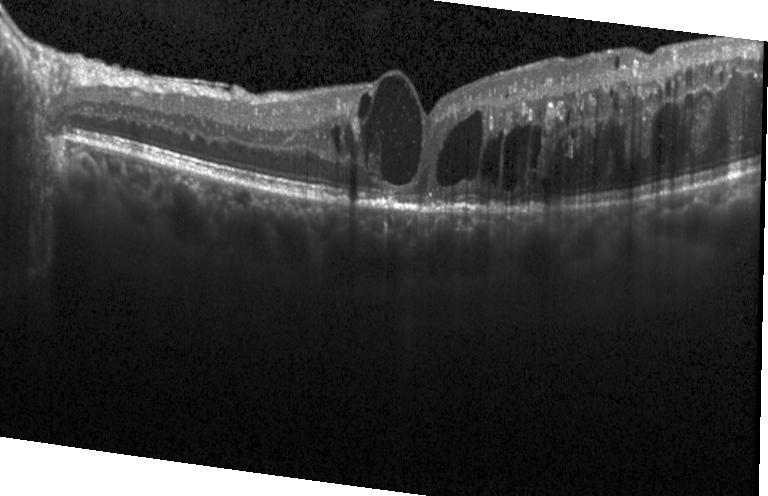 OCT B-scan; horizontal scan through the fovea
Macular OCT: diabetic macular edema.